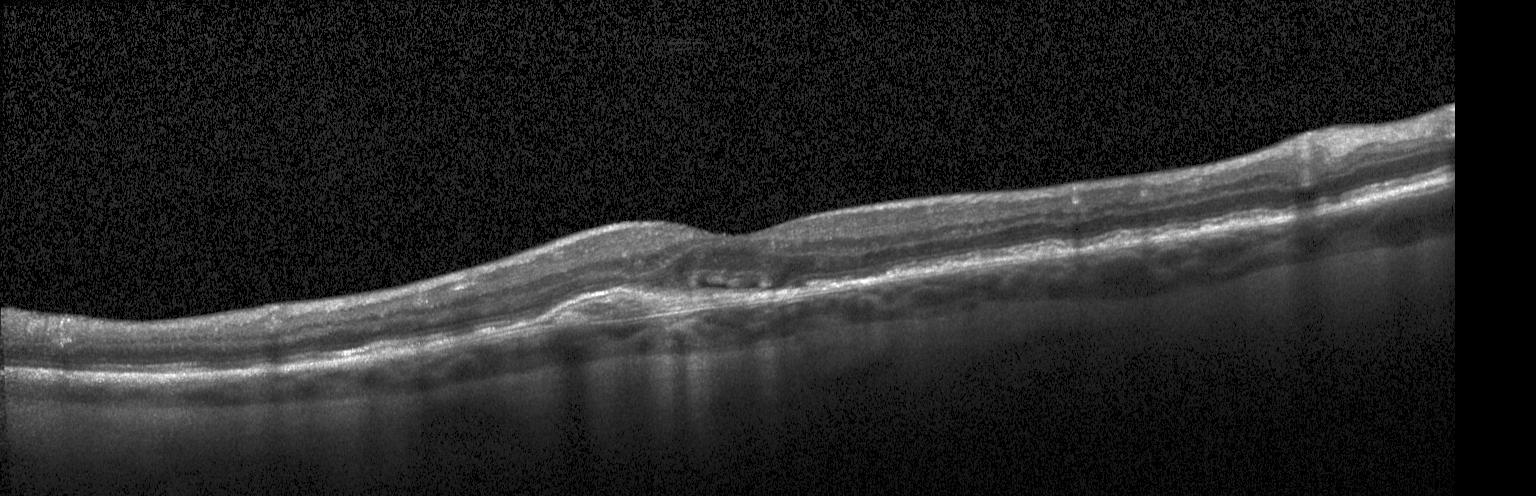 Acquired on a Heidelberg Spectralis. Retinal OCT cross-section. Spectral-domain OCT. Fovea-centered. The scan shows choroidal neovascularization (CNV).